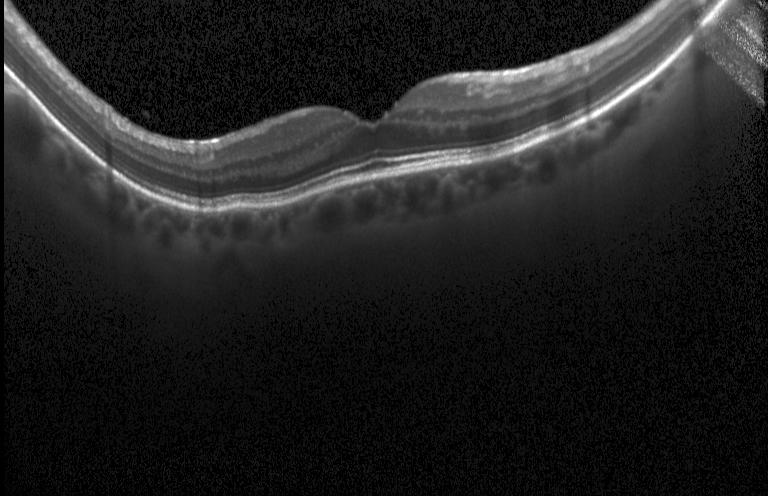 Optical coherence tomography B-scan
Macular OCT: no choroidal neovascularization, diabetic macular edema, or drusen.